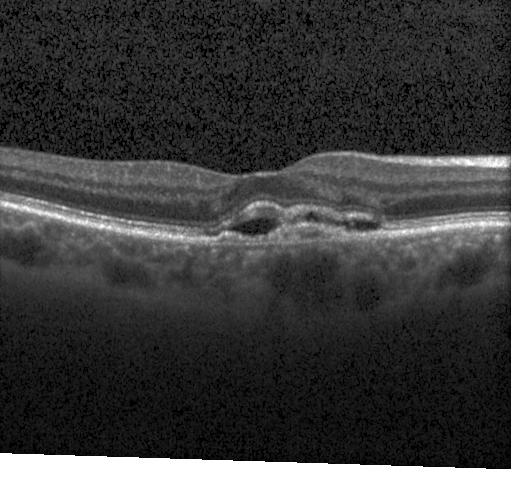
OCT scan showing a choroidal neovascular membrane.